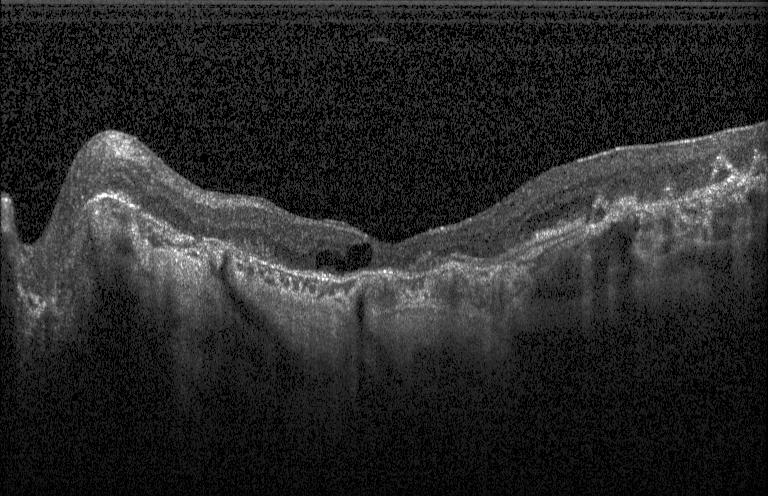

Optical coherence tomography scan.
Choroidal neovascularization.